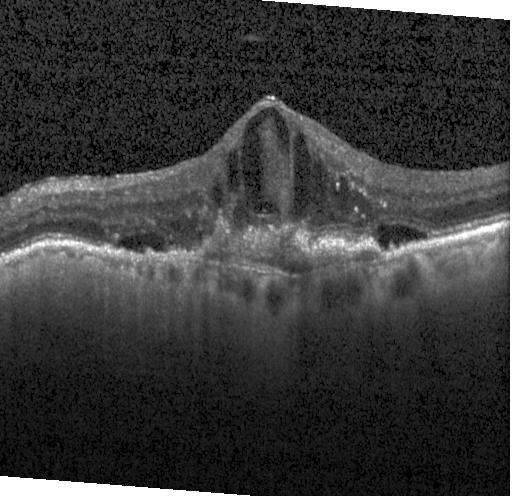

Assessment: a choroidal neovascular membrane.